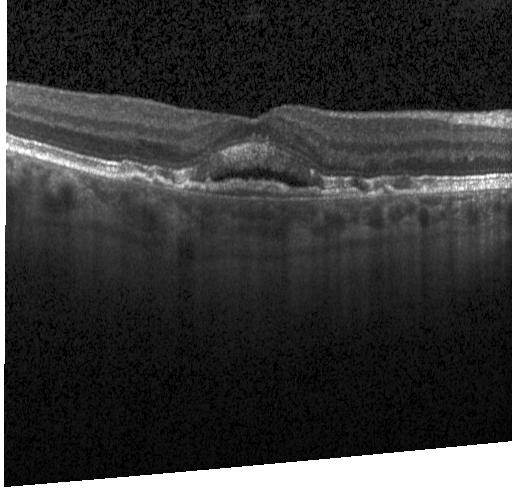 Dx: choroidal neovascularization (CNV).